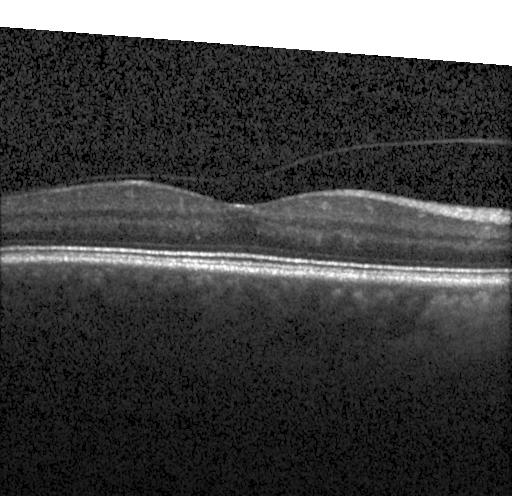
Optical coherence tomography scan, instrument: Heidelberg Spectralis, spectral-domain optical coherence tomography
Finding: no evidence of choroidal neovascularization, diabetic macular edema, or drusen.